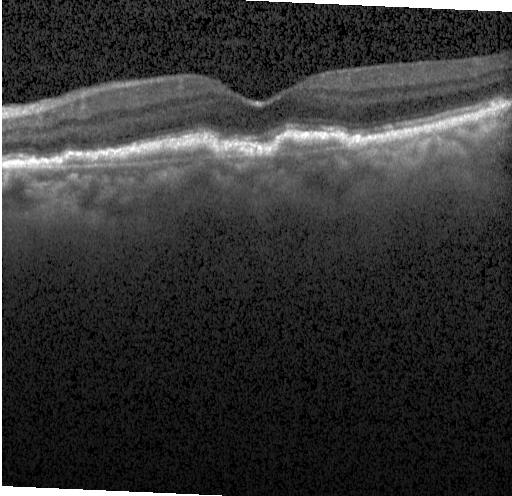
This B-scan demonstrates choroidal neovascularization (CNV).